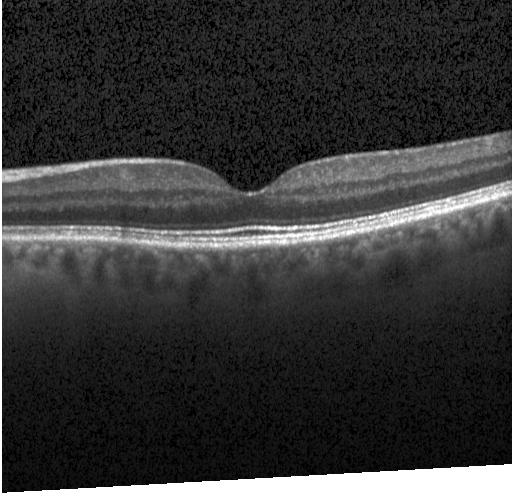
Retinal OCT cross-section showing neither choroidal neovascularization, diabetic macular edema, nor drusen.